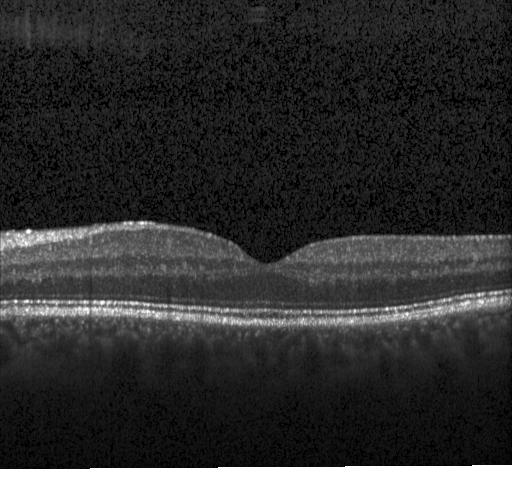

OCT scan showing neither choroidal neovascularization, diabetic macular edema, nor drusen.